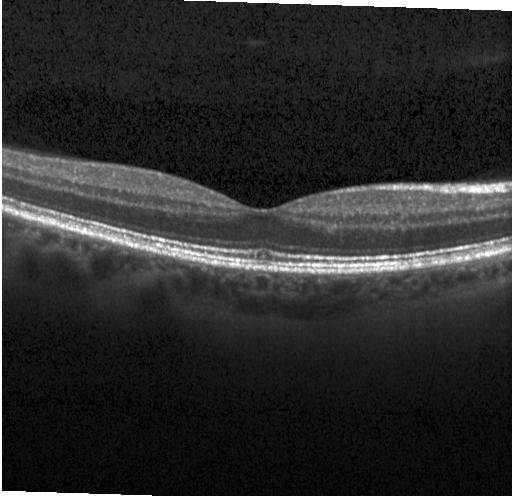

Retinal OCT B-scan. Finding: neither CNV, DME, nor drusen.